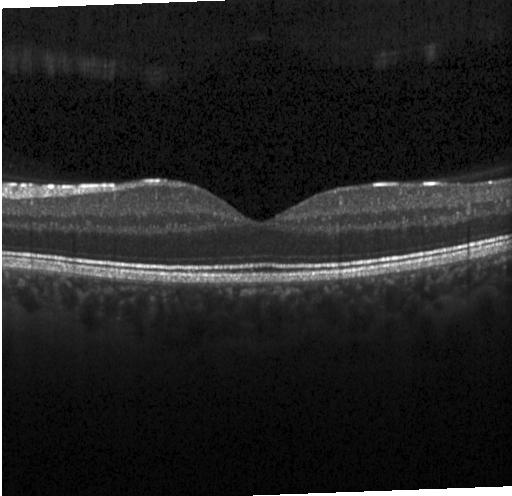
OCT line scan · centered on the fovea
Dx: no evidence of choroidal neovascularization, diabetic macular edema, or drusen.